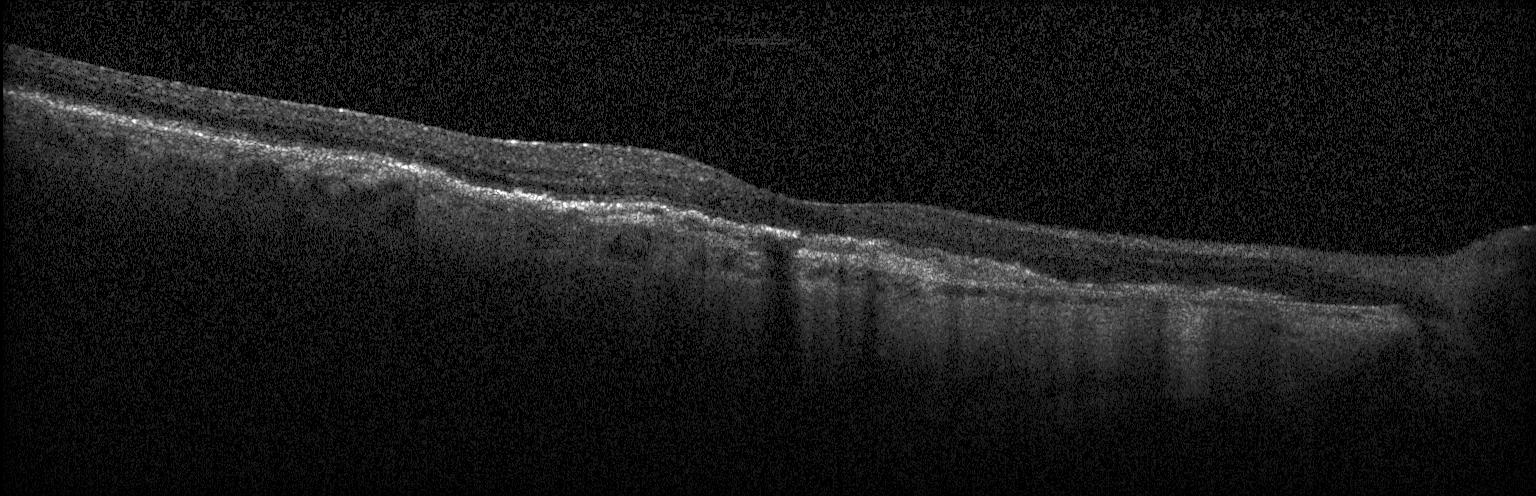

Spectral-domain OCT · optical coherence tomography scan
Finding: choroidal neovascularization (CNV).